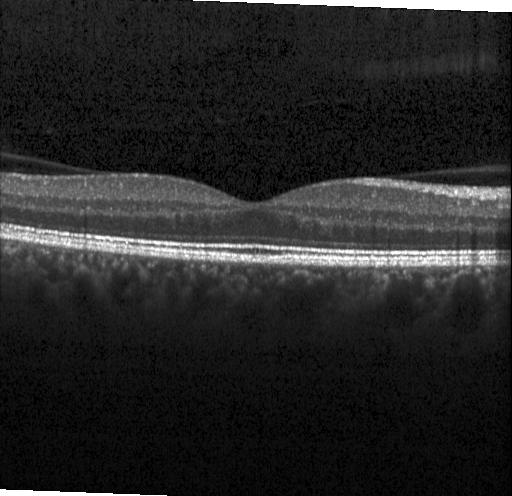

Macular OCT demonstrating no CNV, no DME, and no drusen.